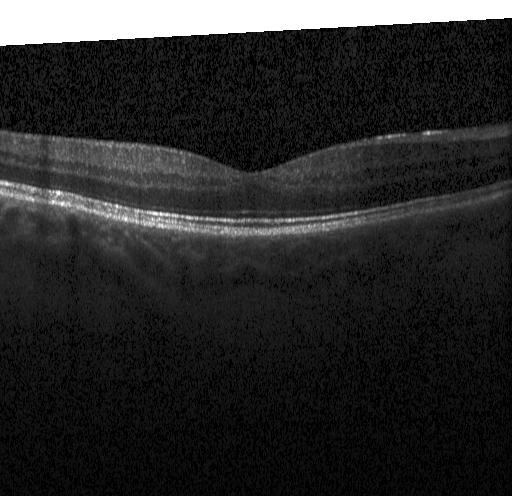 Horizontal scan through the fovea · optical coherence tomography B-scan.
OCT finding: no choroidal neovascularization, diabetic macular edema, or drusen.